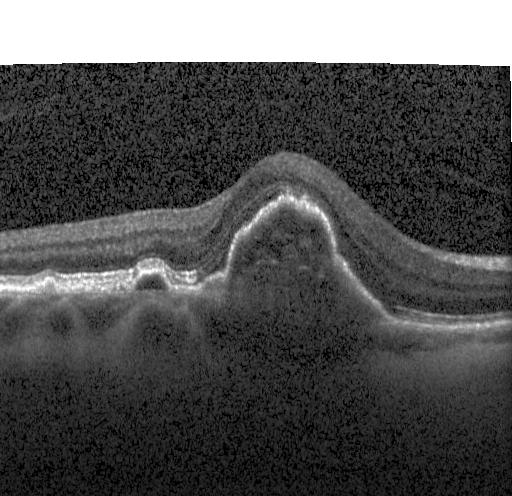
Instrument: Heidelberg Spectralis, SD-OCT, OCT B-scan, fovea-centered — Finding: choroidal neovascularization (CNV).